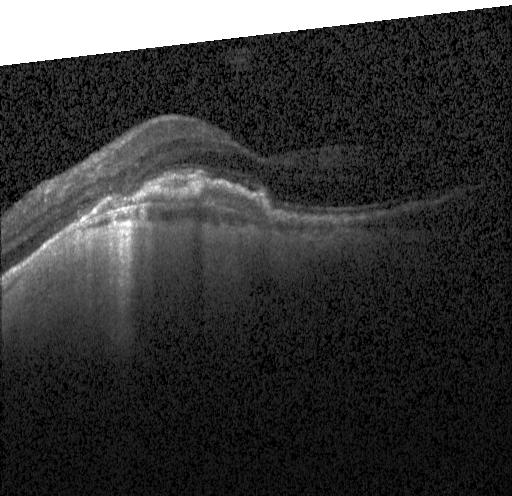

Instrument: Heidelberg Spectralis, OCT B-scan
Diagnosis: a choroidal neovascular membrane.